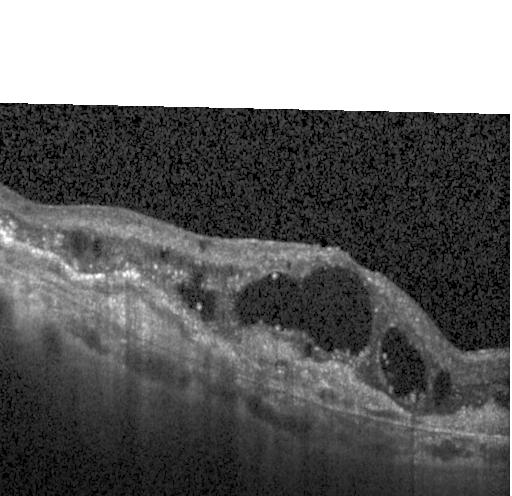

Retinal OCT B-scan. Through the macula. Heidelberg Spectralis.
Assessment: choroidal neovascularization.